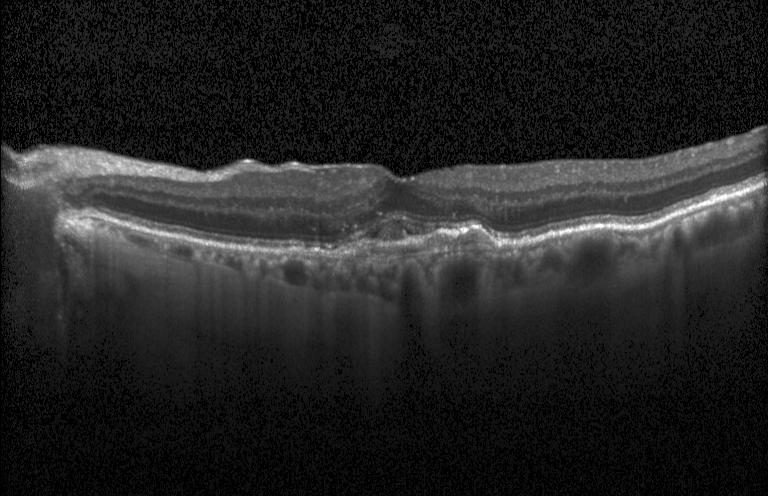 Impression: choroidal neovascularization (CNV).